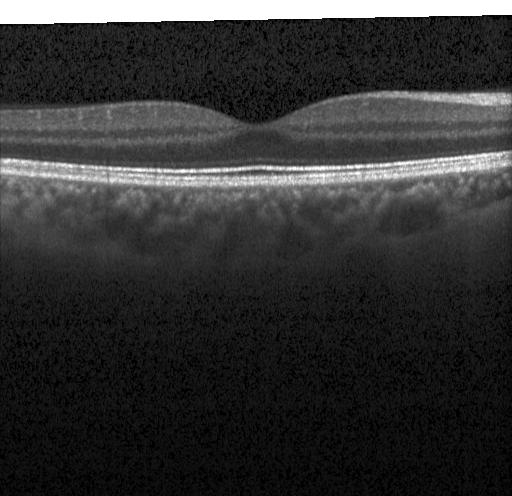

Through the macula; retinal OCT B-scan; acquired on a Heidelberg Spectralis; spectral-domain optical coherence tomography. The scan shows neither choroidal neovascularization, diabetic macular edema, nor drusen.